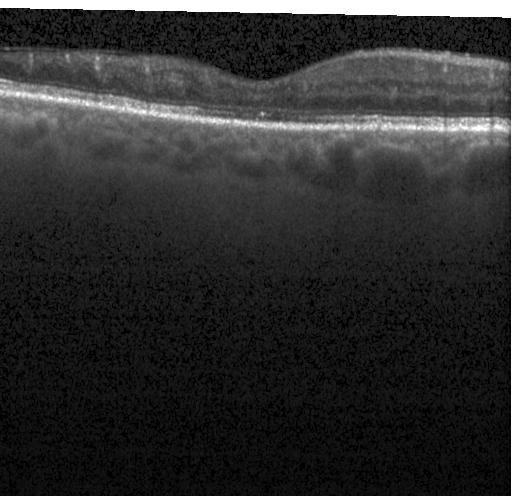

Impression: no evidence of choroidal neovascularization, diabetic macular edema, or drusen.